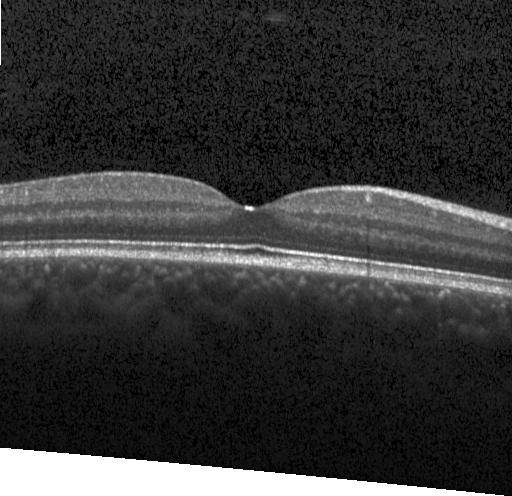

Retinal OCT B-scan.
Macular OCT: no choroidal neovascularization, diabetic macular edema, or drusen.